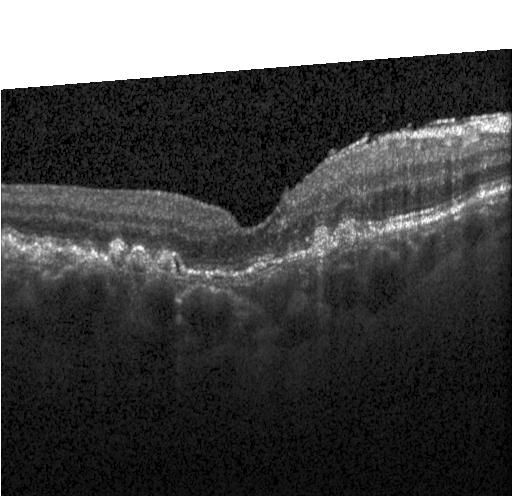 OCT line scan · fovea-centered — Macular OCT: CNV.